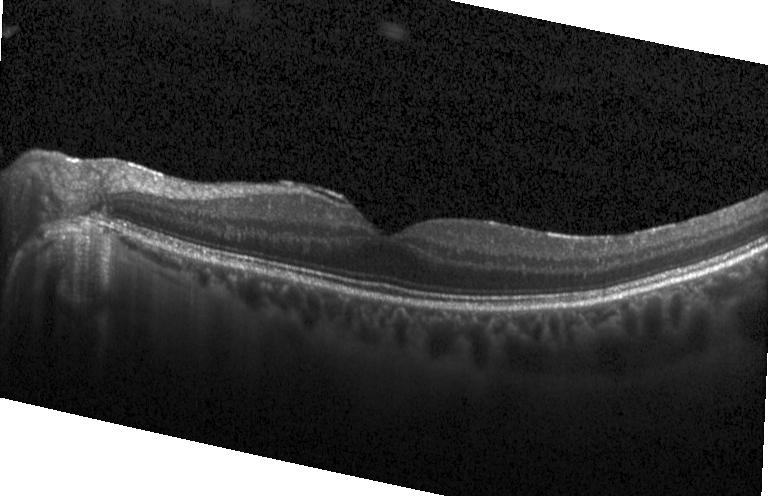
Optical coherence tomography scan. Assessment: no choroidal neovascularization, no diabetic macular edema, and no drusen.